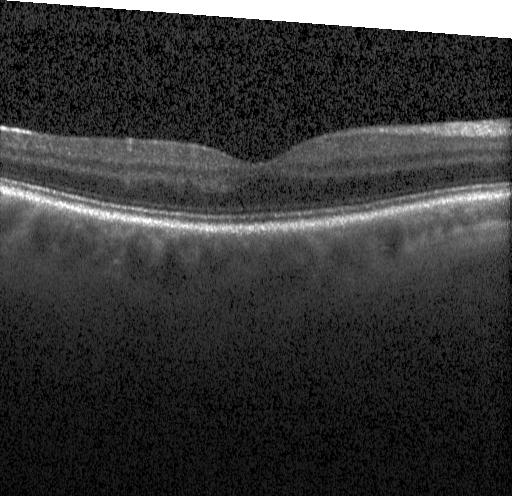
Optical coherence tomography scan. Finding: no CNV, no DME, and no drusen.